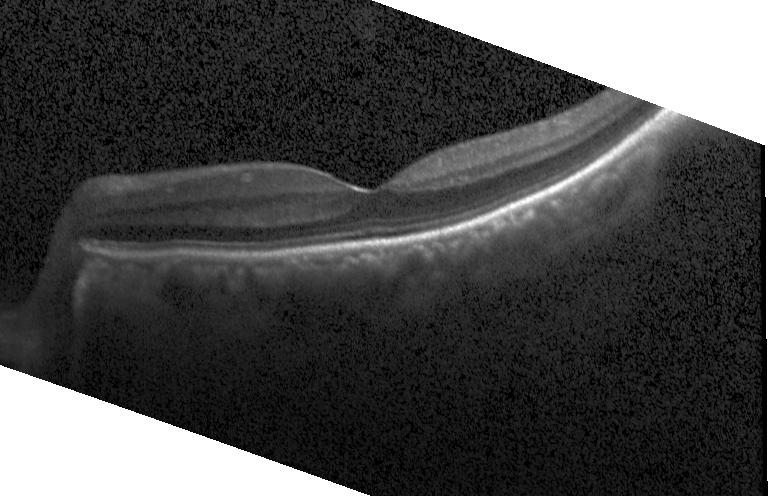 Spectral-domain OCT, fovea-centered, acquired on a Heidelberg Spectralis, OCT B-scan
Finding: neither choroidal neovascularization, diabetic macular edema, nor drusen.